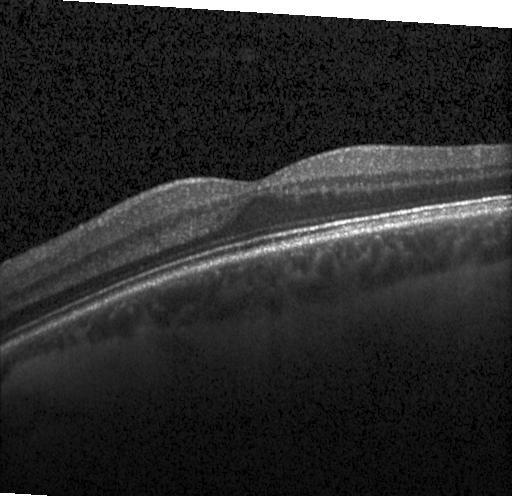 Diagnosis: neither choroidal neovascularization, diabetic macular edema, nor drusen.